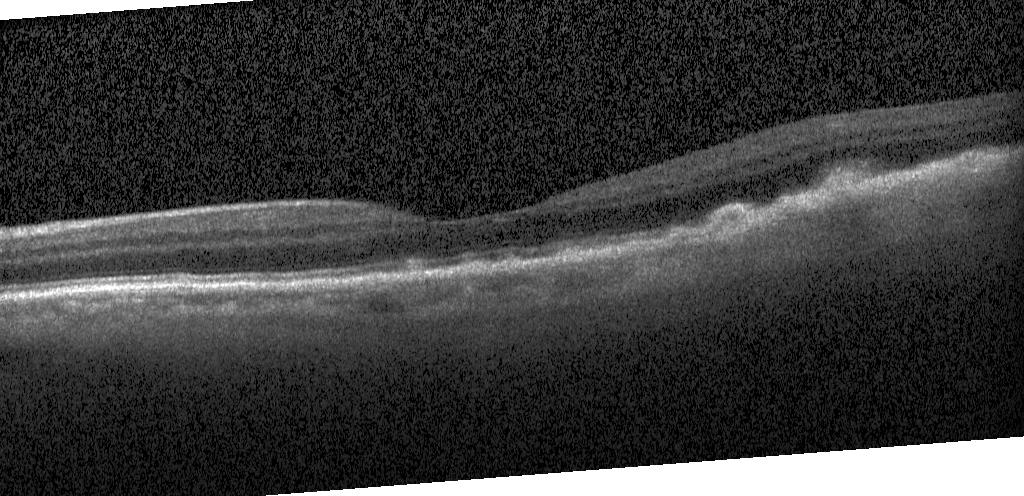

Finding: a choroidal neovascular membrane.